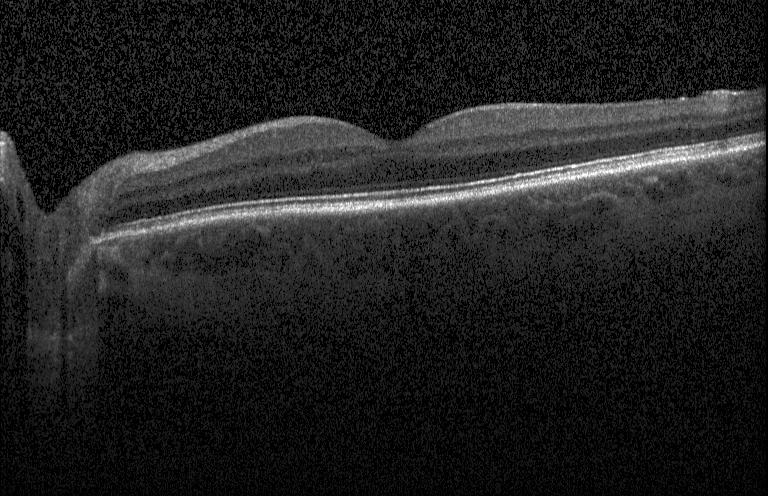 Optical coherence tomography scan. Centered on the fovea — Assessment: no evidence of choroidal neovascularization, diabetic macular edema, or drusen.